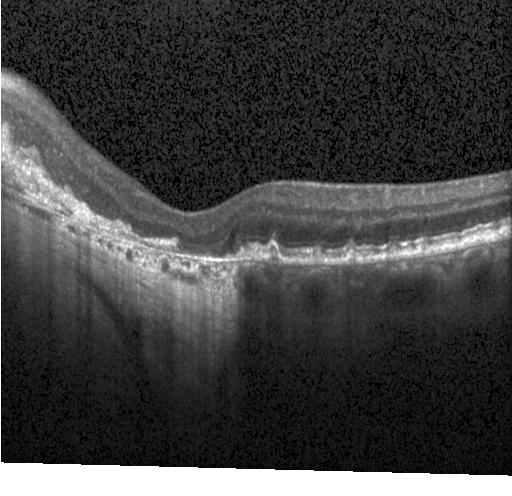
Macular OCT: a choroidal neovascular membrane.